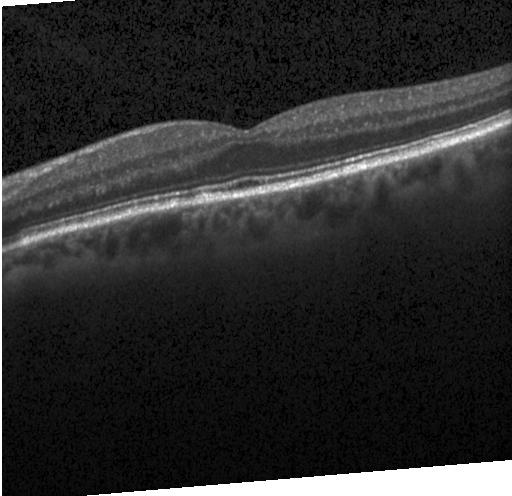
Dx: no evidence of choroidal neovascularization, diabetic macular edema, or drusen.